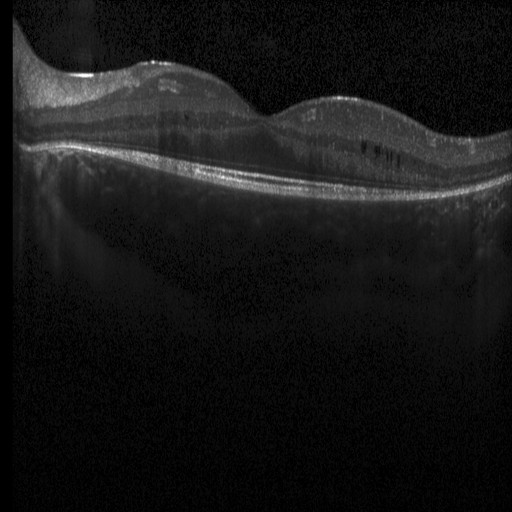
Optical coherence tomography scan · spectral-domain OCT · Heidelberg Spectralis OCT system · through the macula. OCT finding: diabetic macular edema.